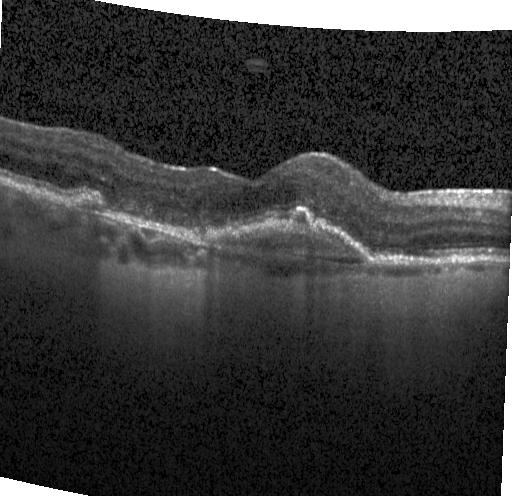 This B-scan demonstrates a choroidal neovascular membrane.